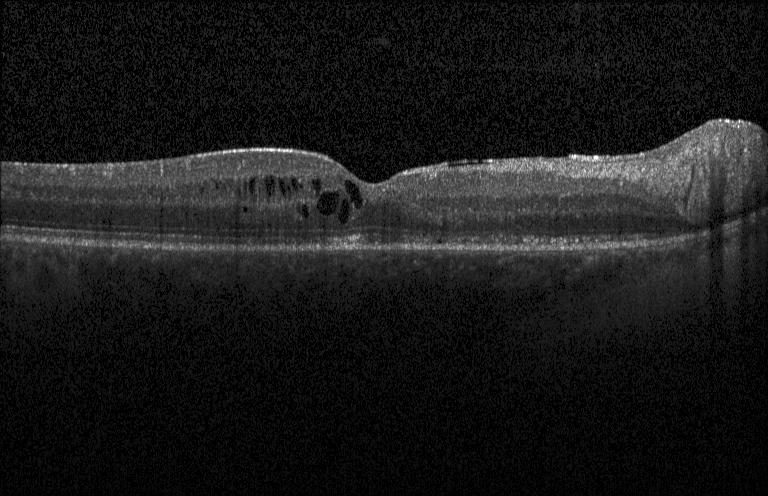

Assessment: DME.